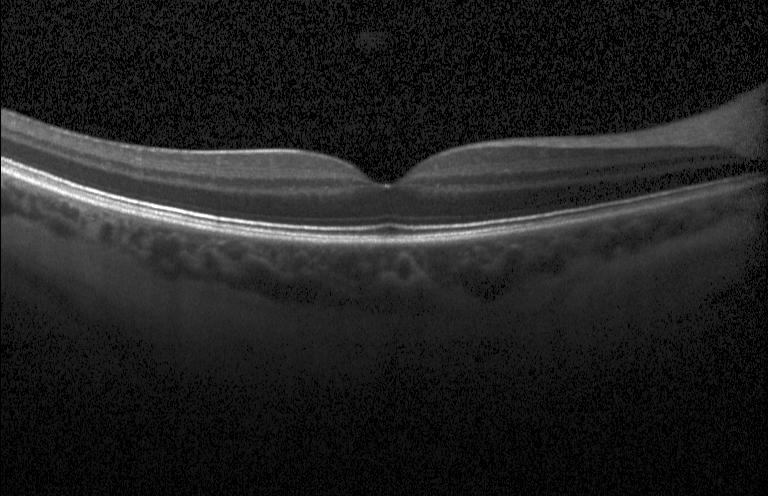 Assessment: no evidence of choroidal neovascularization, diabetic macular edema, or drusen.